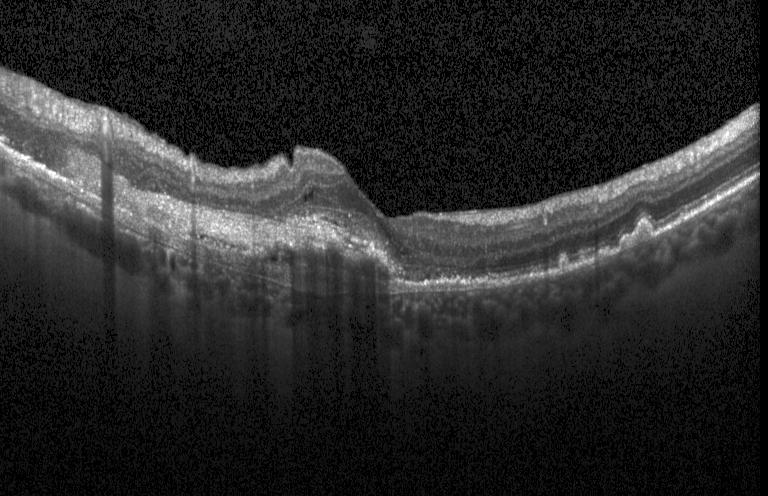
Dx: choroidal neovascularization.